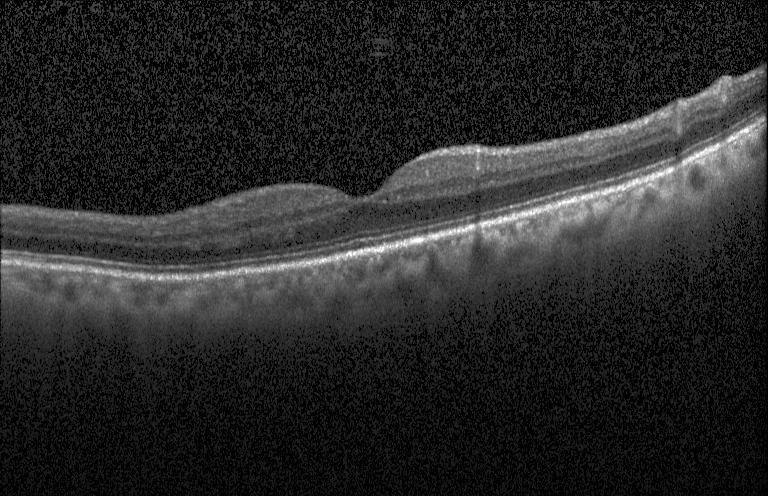
SD-OCT. Heidelberg Spectralis. Retinal OCT cross-section.
No CNV, no DME, and no drusen.